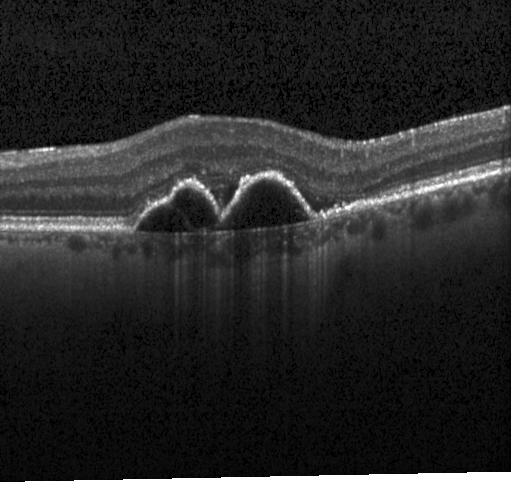

OCT B-scan; Heidelberg Spectralis; centered on the fovea — Finding: choroidal neovascularization.